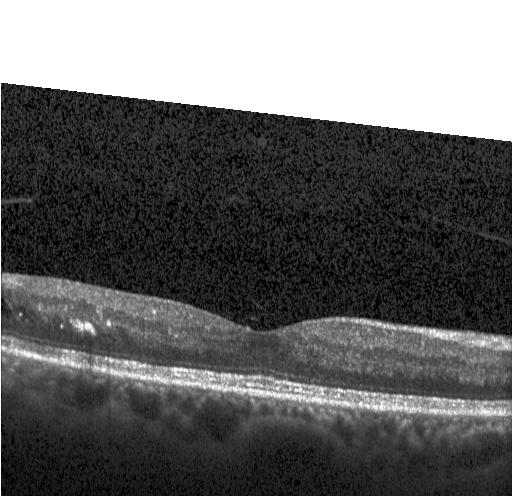 Acquired on a Heidelberg Spectralis. Through the macula. OCT line scan
Diagnosis: diabetic macular edema.